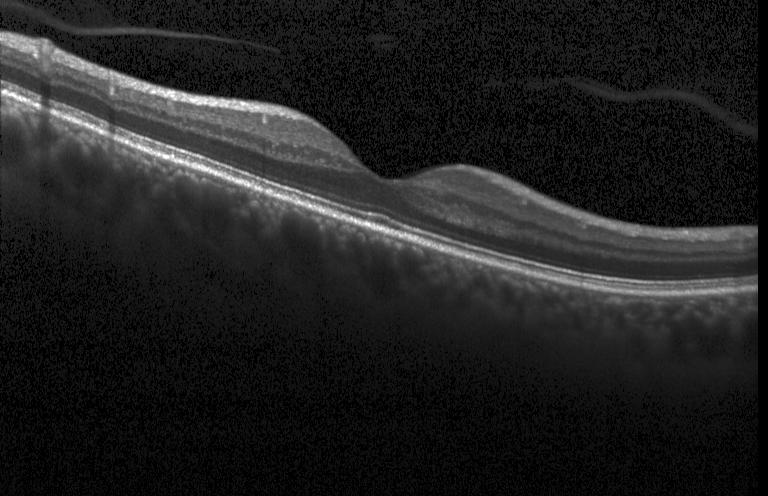

Retinal OCT cross-section showing neither CNV, DME, nor drusen.